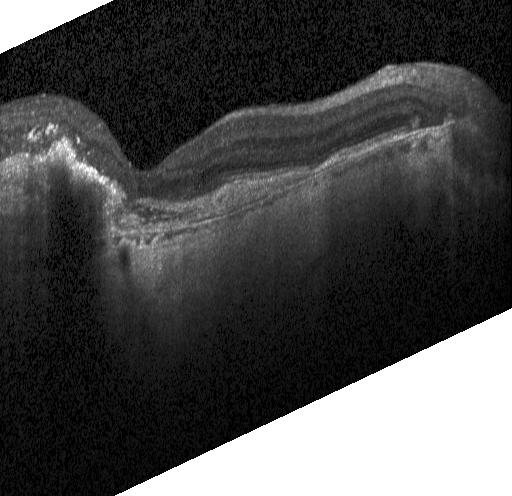 Diagnosis: a choroidal neovascular membrane.